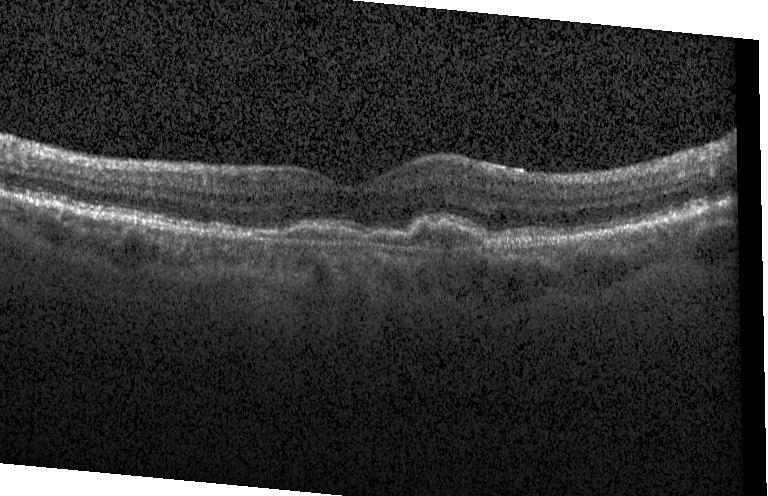

OCT line scan · spectral-domain optical coherence tomography · horizontal scan through the fovea
Diagnosis: choroidal neovascularization.